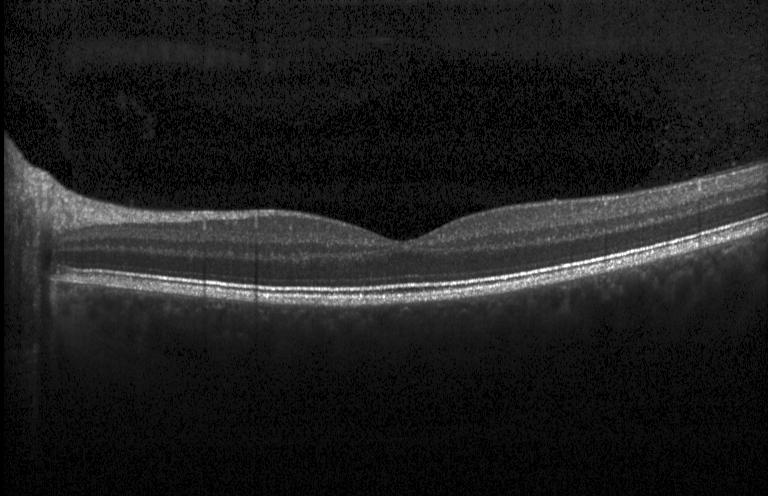
OCT B-scan.
Impression: no evidence of choroidal neovascularization, diabetic macular edema, or drusen.